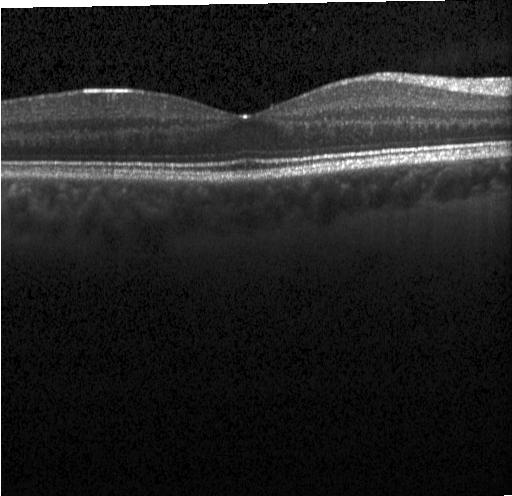
This B-scan demonstrates no evidence of CNV, DME, or drusen.